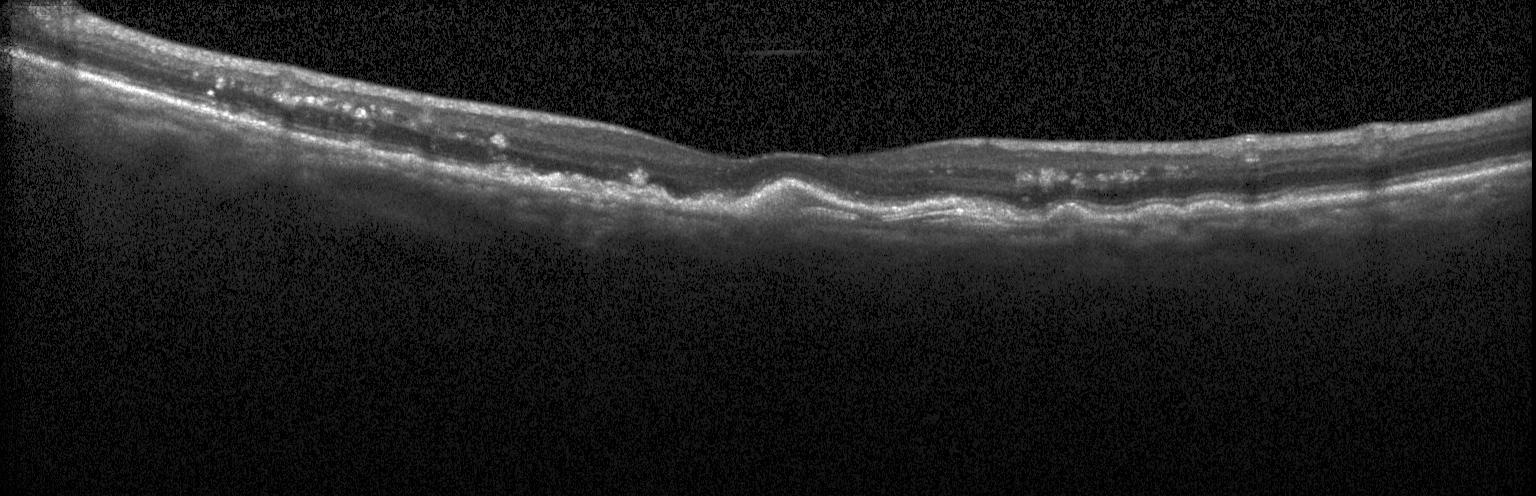 Optical coherence tomography scan.
Dx: a choroidal neovascular membrane.